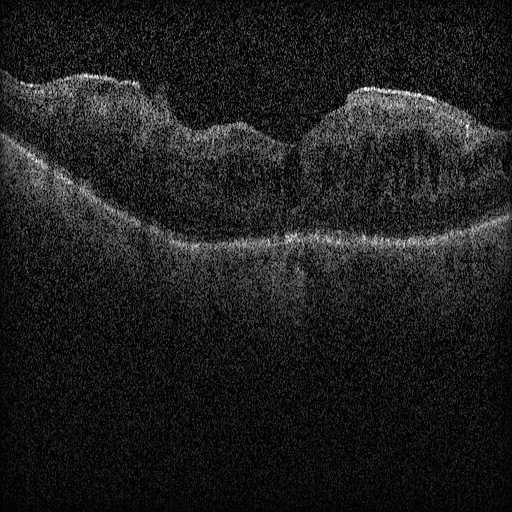
Finding: diabetic macular edema (DME).